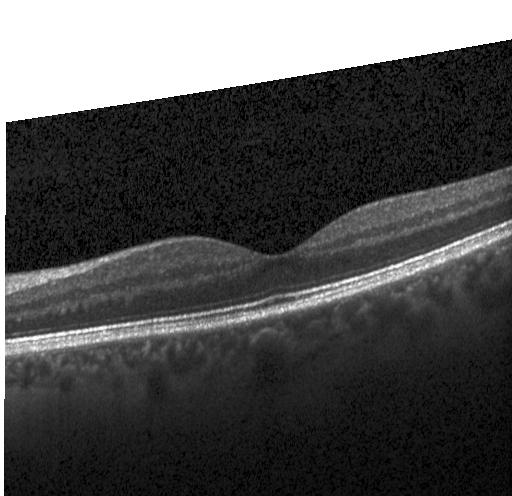

OCT scan showing no choroidal neovascularization, diabetic macular edema, or drusen.